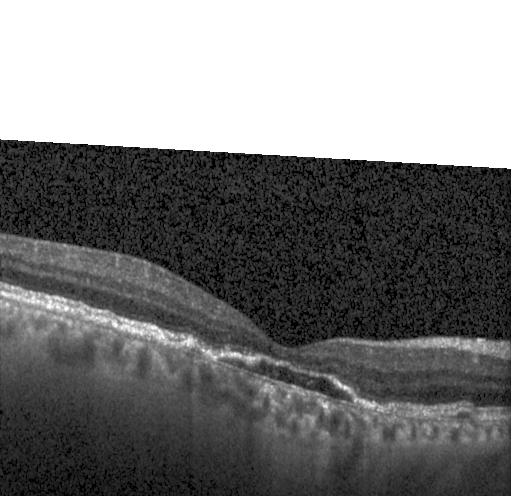

Retinal OCT cross-section showing a choroidal neovascular membrane.